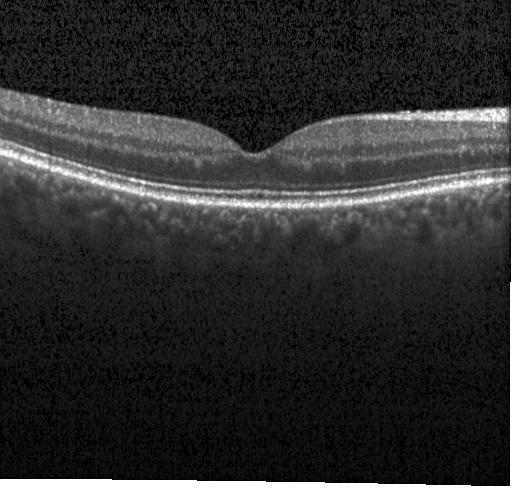
OCT line scan; Heidelberg Spectralis; SD-OCT. Macular OCT: no CNV, DME, or drusen.